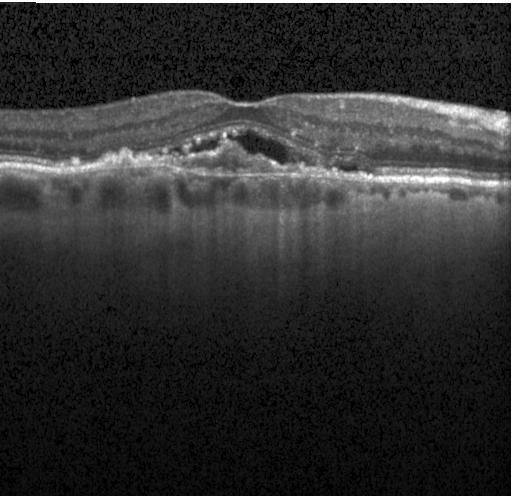
Diagnosis: a choroidal neovascular membrane.